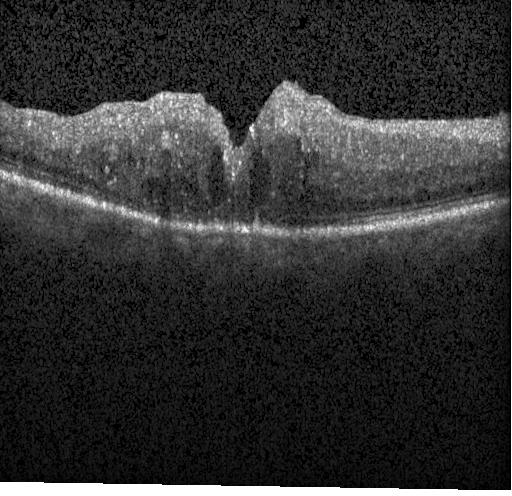

OCT B-scan. Spectral-domain OCT.
OCT finding: diabetic macular edema (DME).